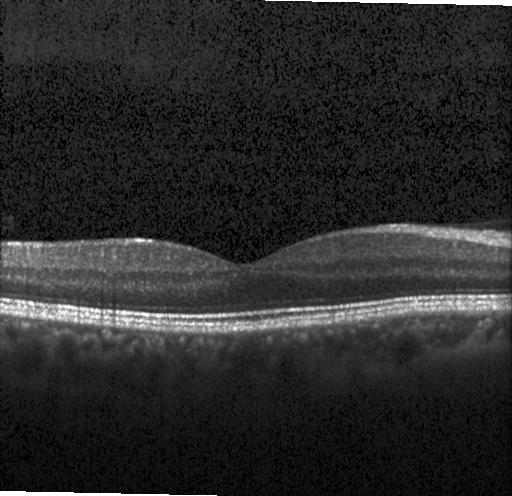
Macular scan · spectral-domain optical coherence tomography · OCT B-scan.
Impression: no choroidal neovascularization, no diabetic macular edema, and no drusen.